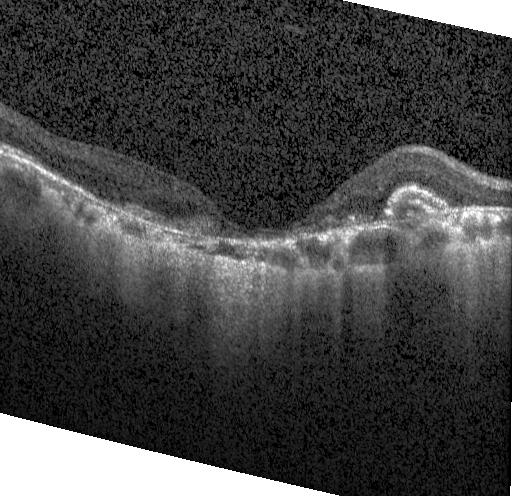
Centered on the fovea. SD-OCT. Retinal OCT cross-section. Heidelberg Spectralis OCT system.
Dx: a choroidal neovascular membrane.